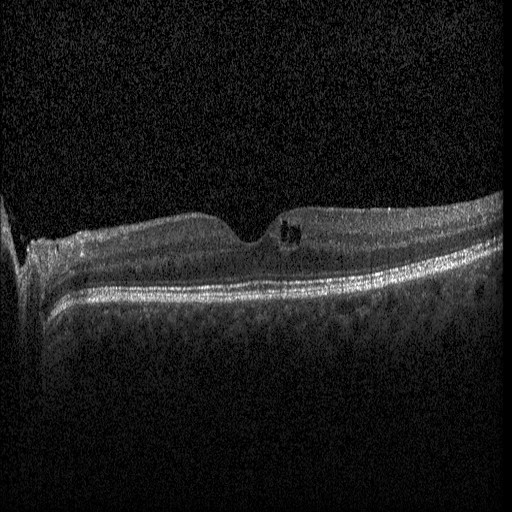 Spectral-domain OCT · instrument: Heidelberg Spectralis · retinal OCT B-scan · horizontal scan through the fovea. This B-scan demonstrates diabetic macular edema (DME).